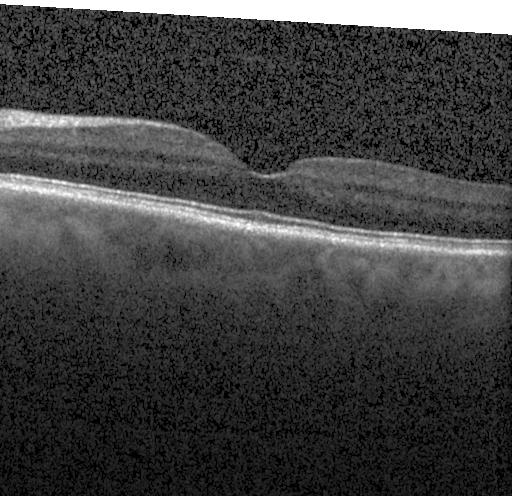
Through the macula. Retinal OCT B-scan. Heidelberg Spectralis — Assessment: no choroidal neovascularization, diabetic macular edema, or drusen.